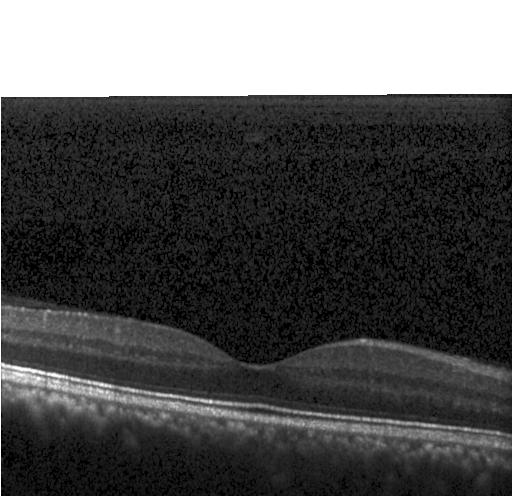 Retinal OCT cross-section. OCT finding: no evidence of choroidal neovascularization, diabetic macular edema, or drusen.